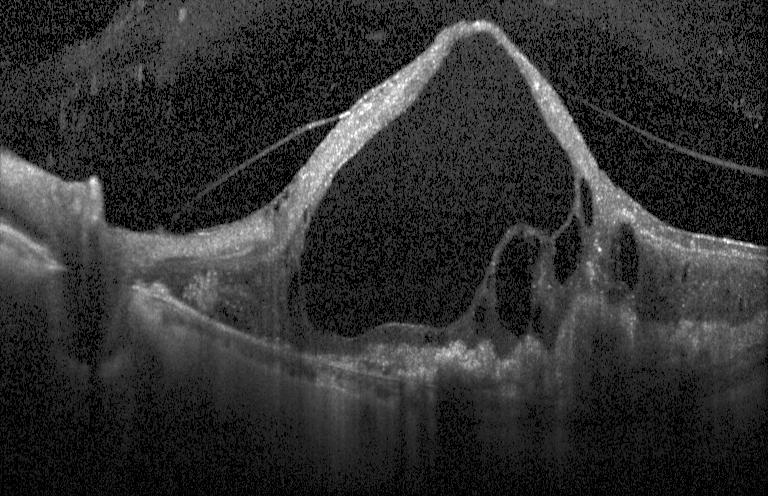

Centered on the fovea · spectral-domain optical coherence tomography · retinal OCT cross-section · Heidelberg Spectralis OCT system — Diagnosis: a choroidal neovascular membrane.